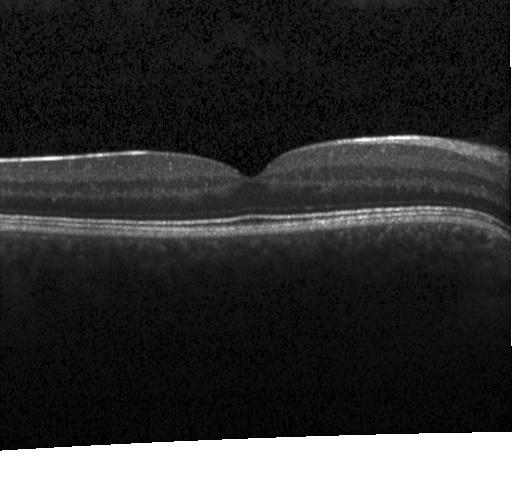

Spectral-domain OCT B-scan: no choroidal neovascularization, no diabetic macular edema, and no drusen.